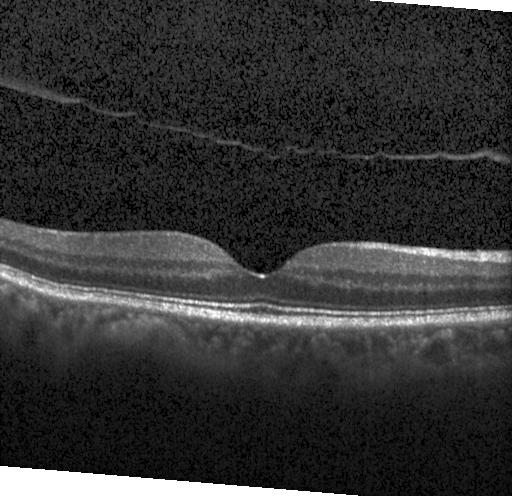 Dx: no choroidal neovascularization, diabetic macular edema, or drusen.